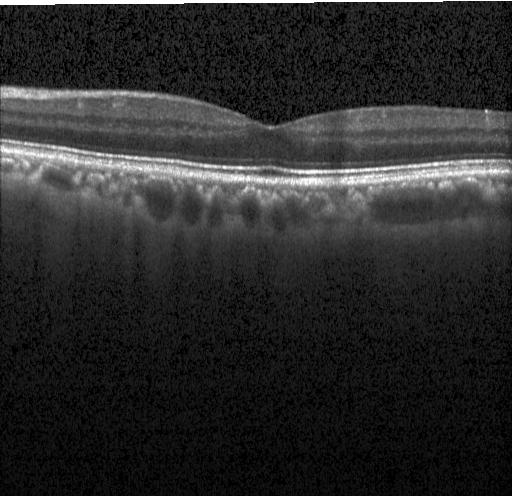 OCT line scan. SD-OCT
Diagnosis: neither choroidal neovascularization, diabetic macular edema, nor drusen.